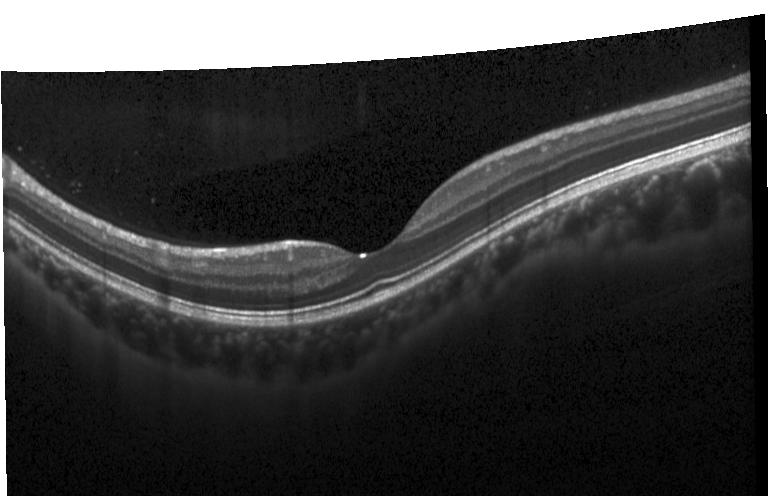
Retinal OCT cross-section, through the macula, Heidelberg Spectralis OCT system
Dx: neither CNV, DME, nor drusen.